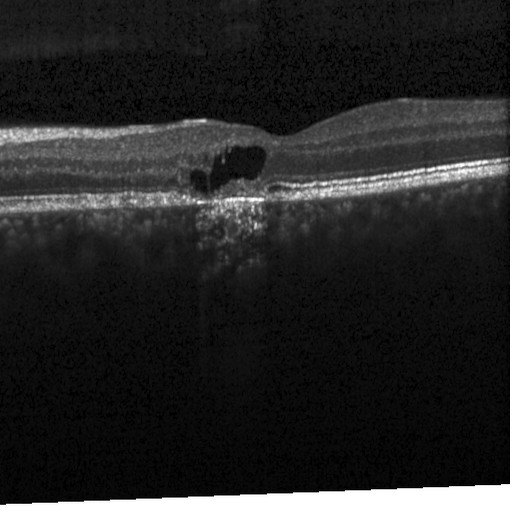 OCT B-scan. Instrument: Heidelberg Spectralis — Assessment: diabetic macular edema (DME).